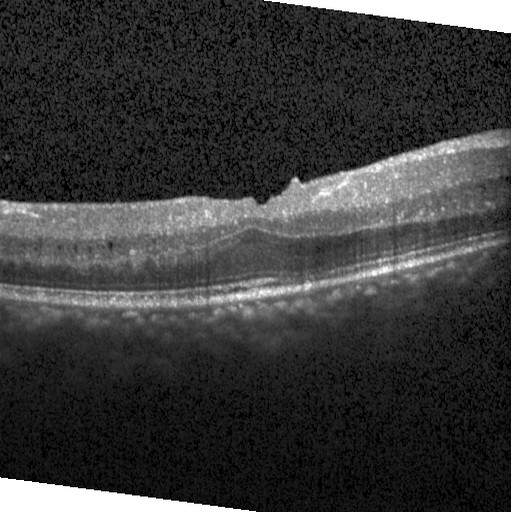

Optical coherence tomography scan — Diagnosis: diabetic macular edema (DME).